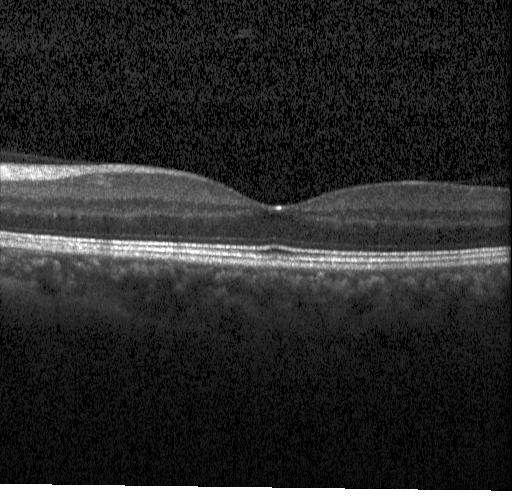 Spectral-domain OCT. Fovea-centered. Acquired on a Heidelberg Spectralis. Optical coherence tomography scan — Impression: no evidence of choroidal neovascularization, diabetic macular edema, or drusen.